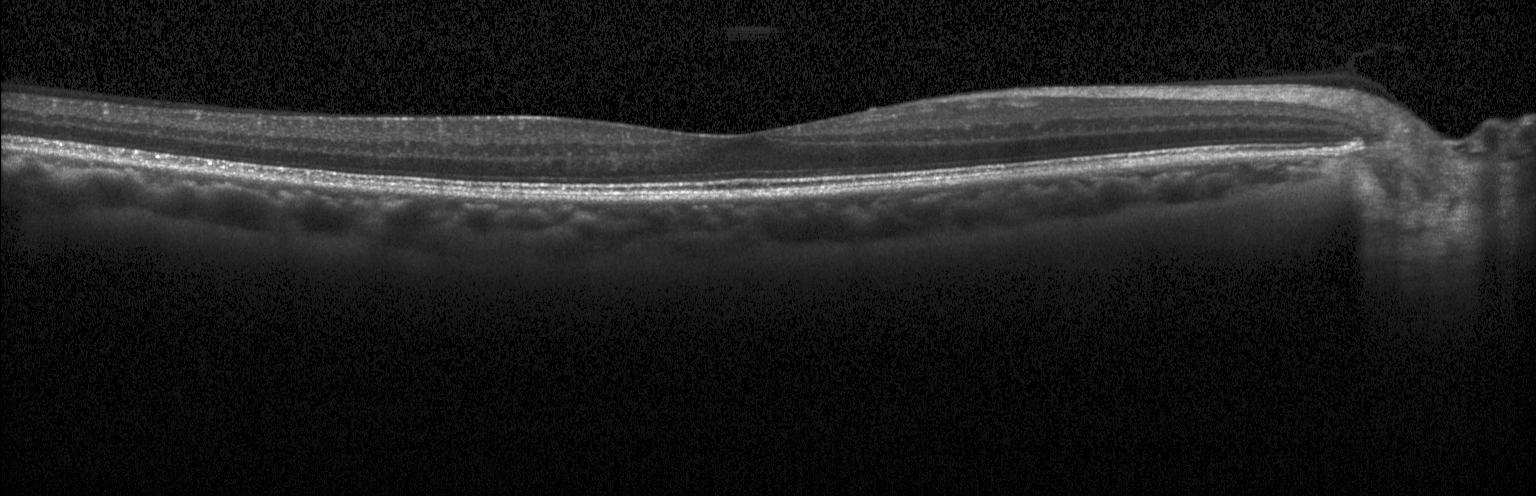 Optical coherence tomography B-scan, horizontal scan through the fovea, instrument: Heidelberg Spectralis — Impression: no evidence of choroidal neovascularization, diabetic macular edema, or drusen.